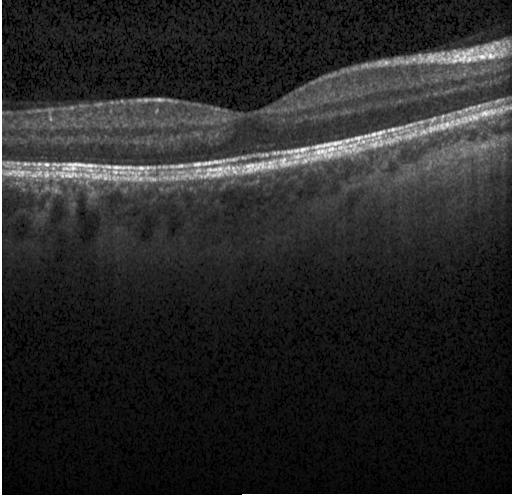
Heidelberg Spectralis; retinal OCT B-scan; macular scan — Diagnosis: no CNV, DME, or drusen.